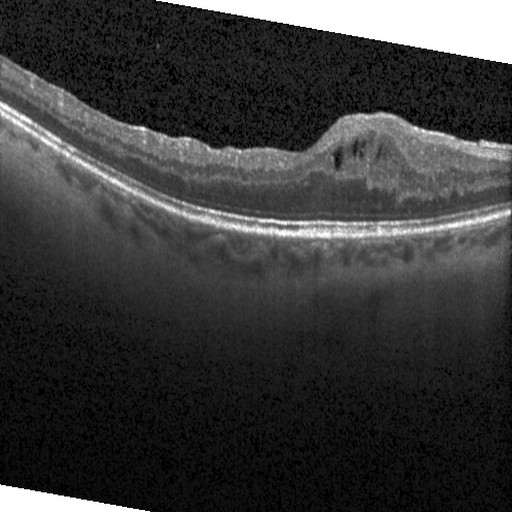
Macular OCT: DME.